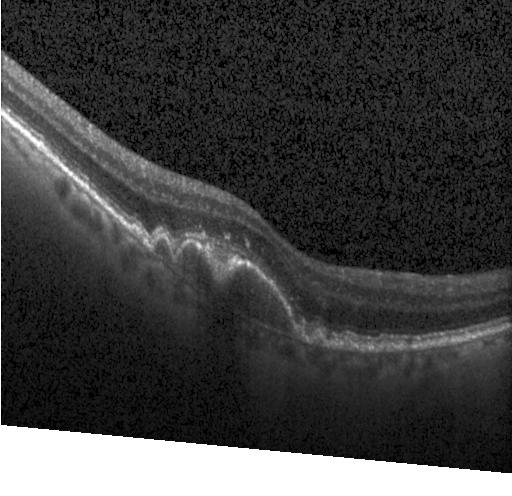 Through the macula; retinal OCT cross-section; acquired on a Heidelberg Spectralis. Assessment: choroidal neovascularization.